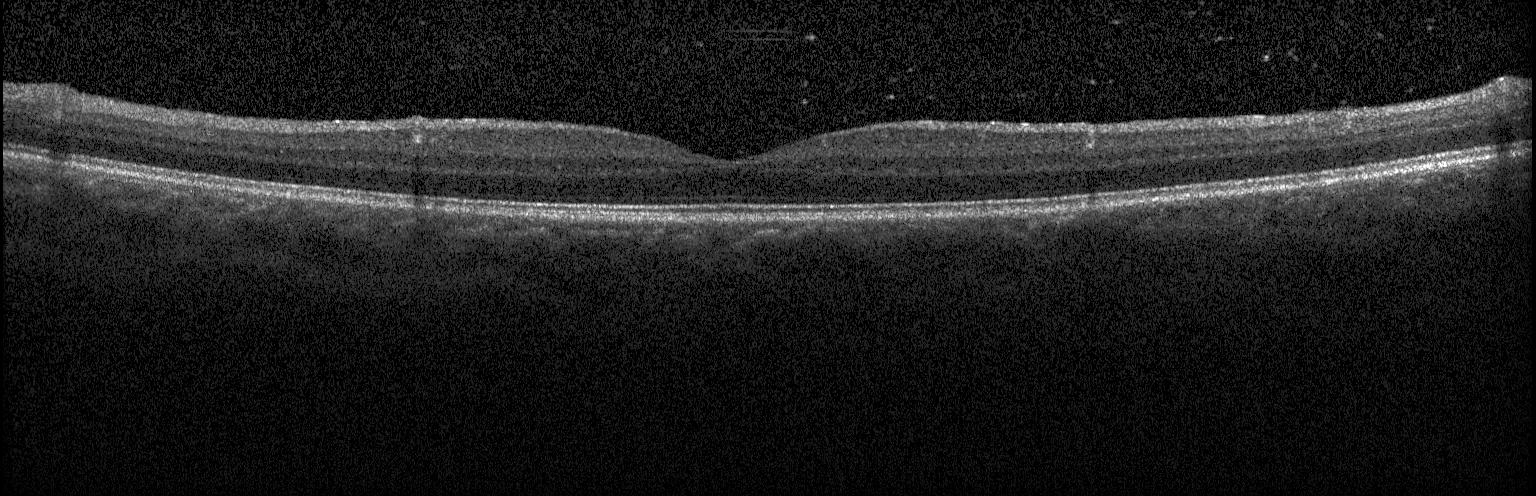 OCT line scan — Diagnosis: no choroidal neovascularization, diabetic macular edema, or drusen.